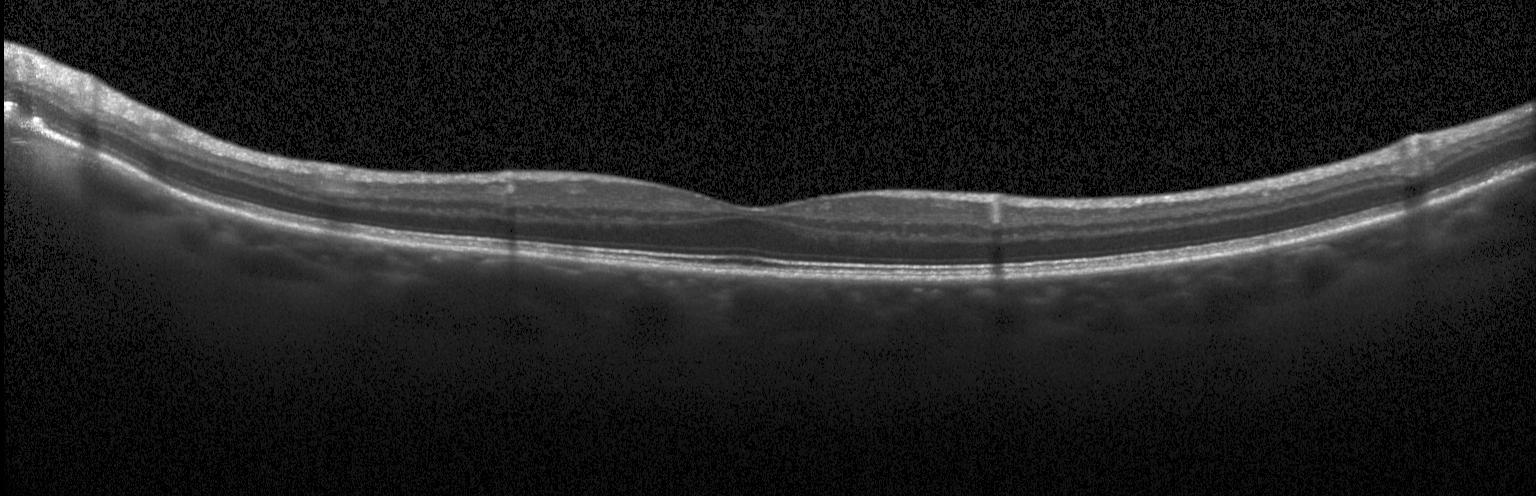
Diagnosis: no evidence of choroidal neovascularization, diabetic macular edema, or drusen.